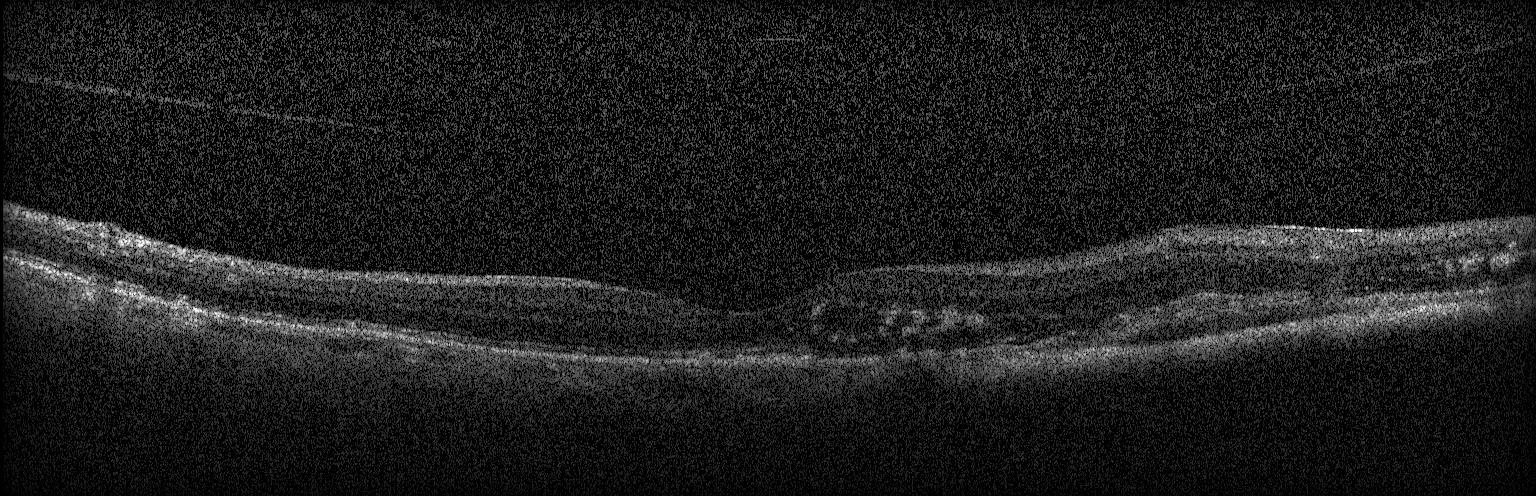
Through the macula; optical coherence tomography B-scan. Finding: choroidal neovascularization (CNV).